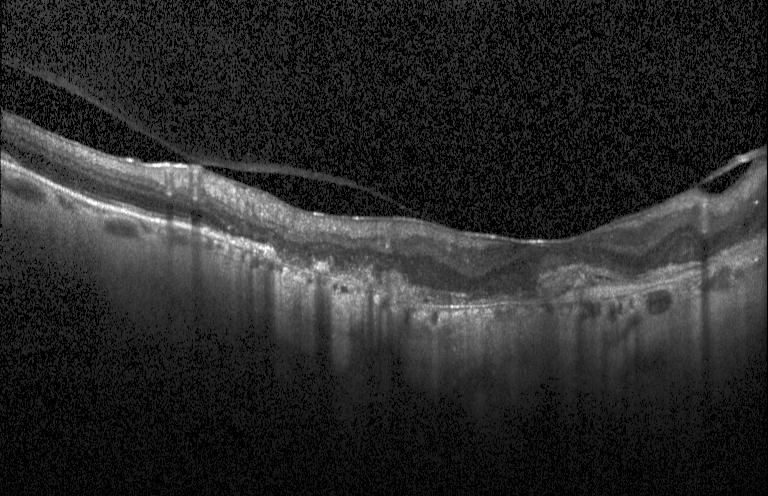

Heidelberg Spectralis, retinal OCT cross-section, centered on the fovea, spectral-domain OCT. Diagnosis: CNV.